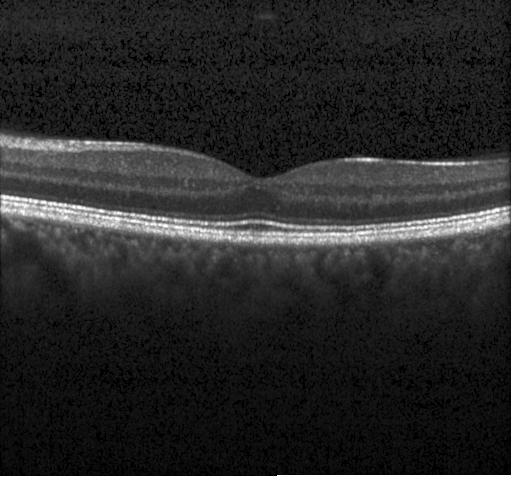
Optical coherence tomography B-scan. Fovea-centered. Acquired on a Heidelberg Spectralis. Dx: no choroidal neovascularization, diabetic macular edema, or drusen.